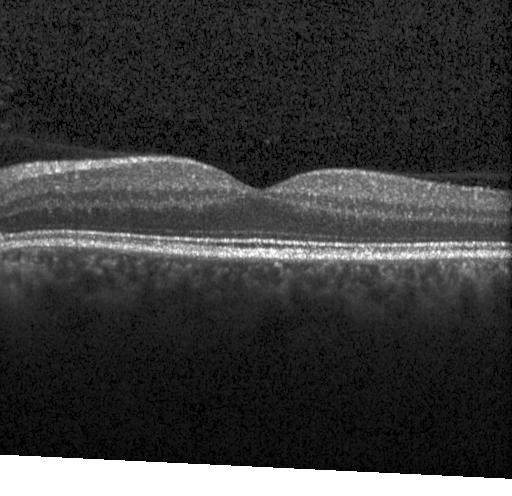 Finding: no evidence of choroidal neovascularization, diabetic macular edema, or drusen.